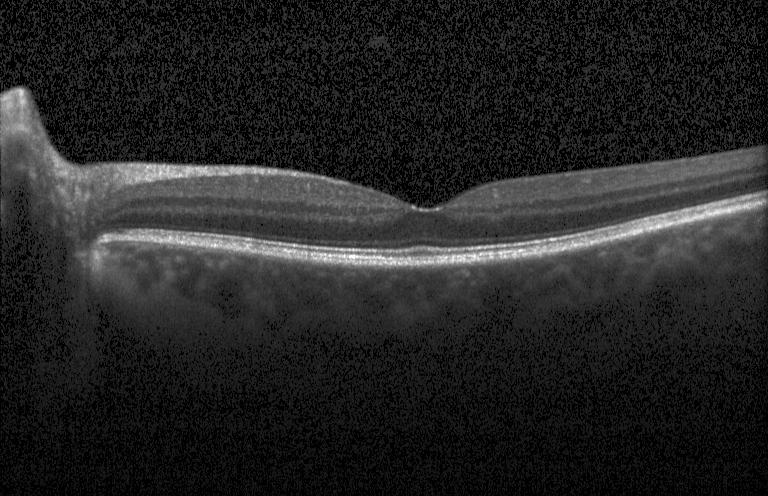
Impression: no choroidal neovascularization, no diabetic macular edema, and no drusen.